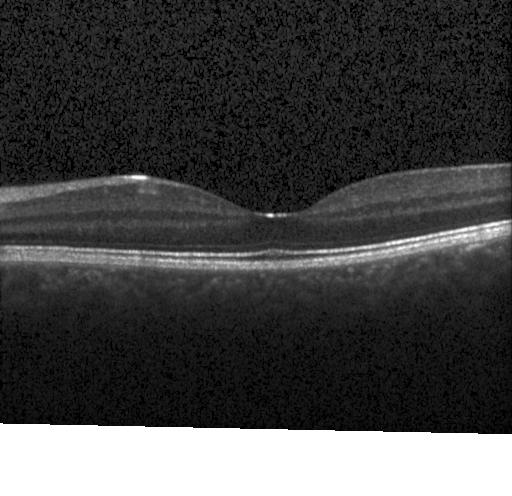
Macular OCT: no evidence of choroidal neovascularization, diabetic macular edema, or drusen.